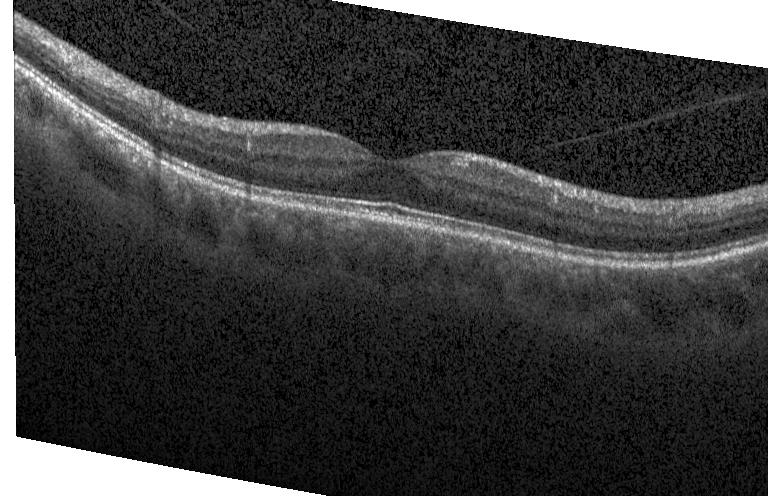

No choroidal neovascularization, no diabetic macular edema, and no drusen.